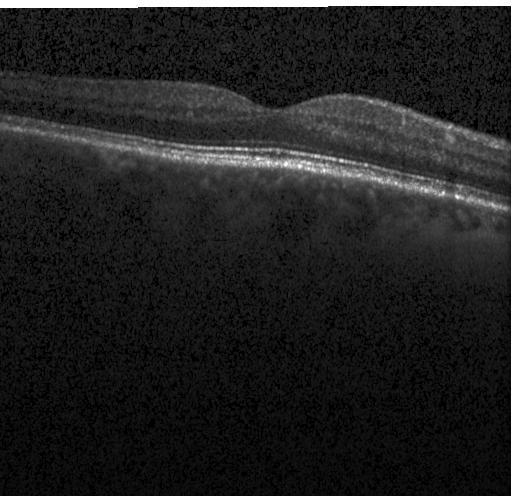 Impression: no choroidal neovascularization, diabetic macular edema, or drusen.